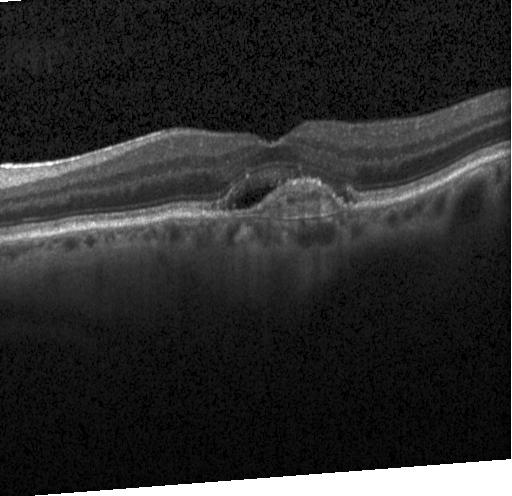 Heidelberg Spectralis OCT system · retinal OCT cross-section · SD-OCT
OCT finding: choroidal neovascularization.